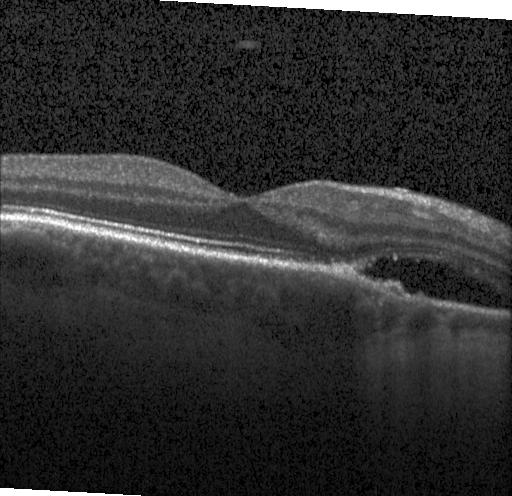

Through the macula · OCT line scan — Assessment: a choroidal neovascular membrane.